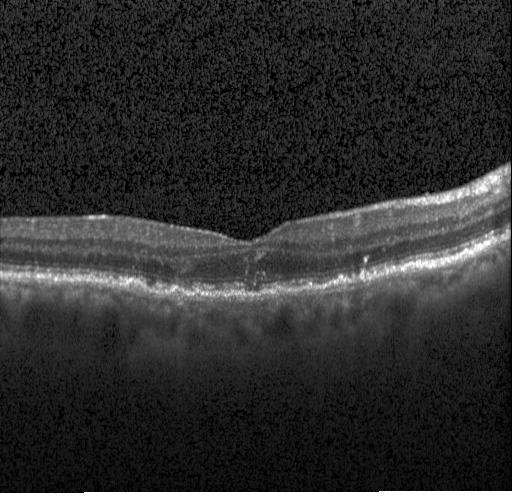
Instrument: Heidelberg Spectralis · retinal OCT B-scan — Assessment: multiple drusen.